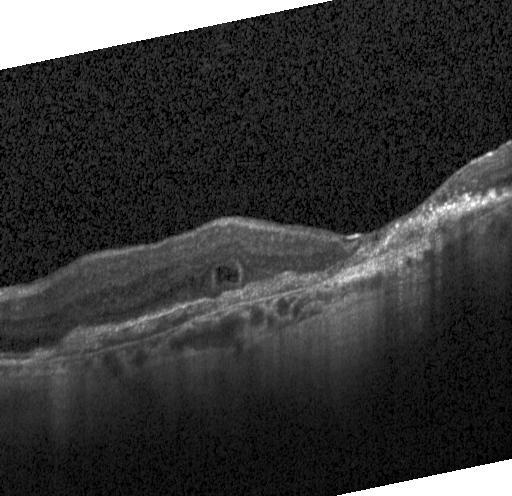 The scan shows choroidal neovascularization.